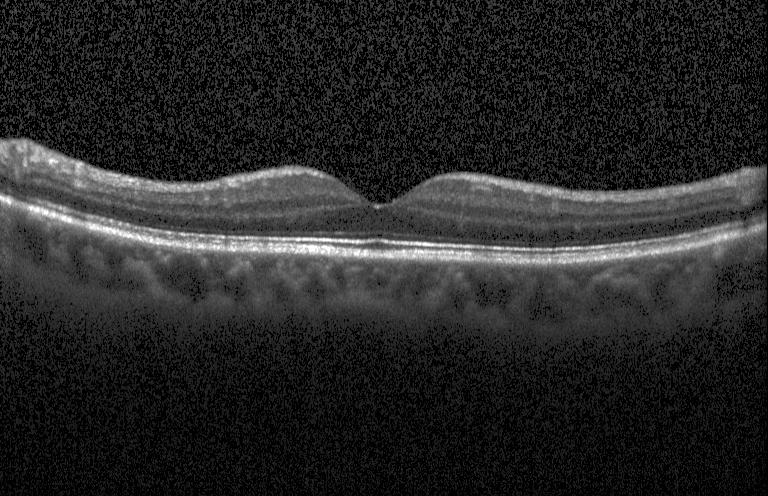
Heidelberg Spectralis, retinal OCT B-scan. Macular OCT: no evidence of choroidal neovascularization, diabetic macular edema, or drusen.